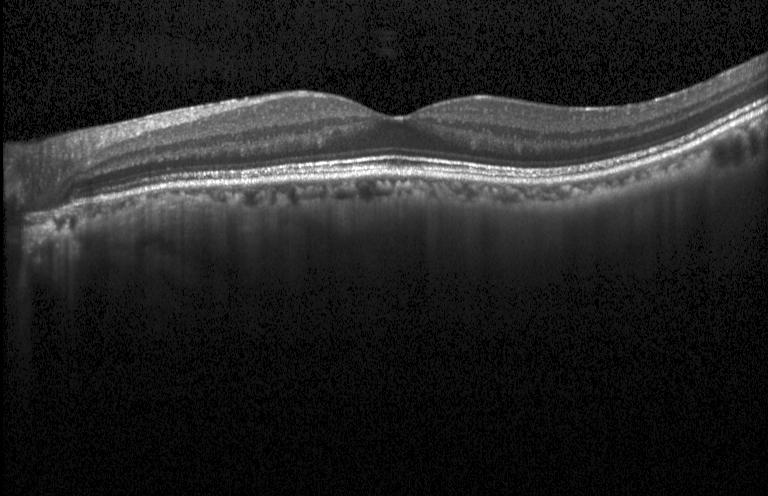 SD-OCT. Retinal OCT cross-section. Instrument: Heidelberg Spectralis
The scan shows no evidence of choroidal neovascularization, diabetic macular edema, or drusen.